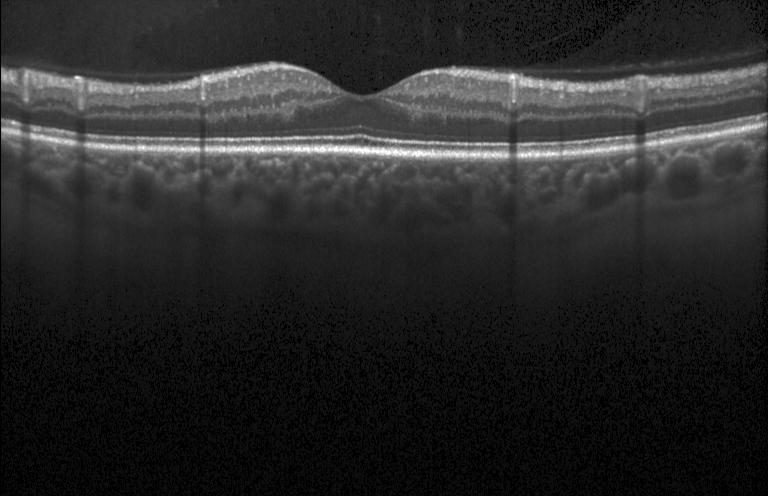

Retinal OCT B-scan.
Macular OCT: no CNV, DME, or drusen.